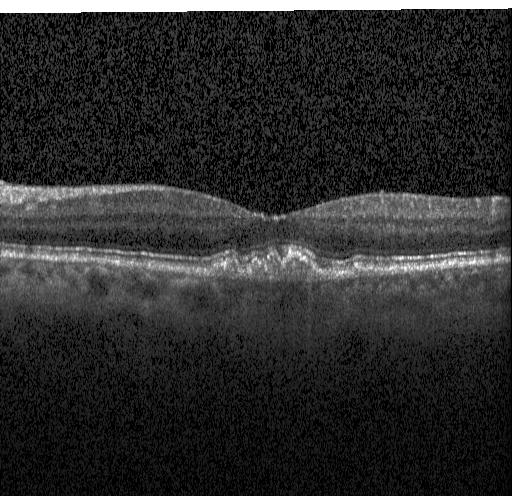 Instrument: Heidelberg Spectralis; spectral-domain optical coherence tomography; centered on the fovea; retinal OCT cross-section. This B-scan demonstrates multiple drusen.